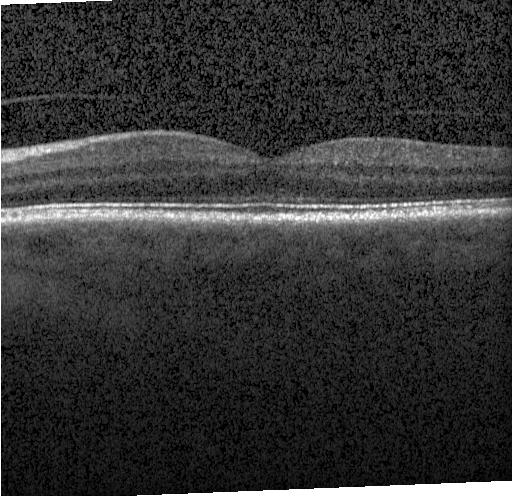 Finding: no evidence of choroidal neovascularization, diabetic macular edema, or drusen.